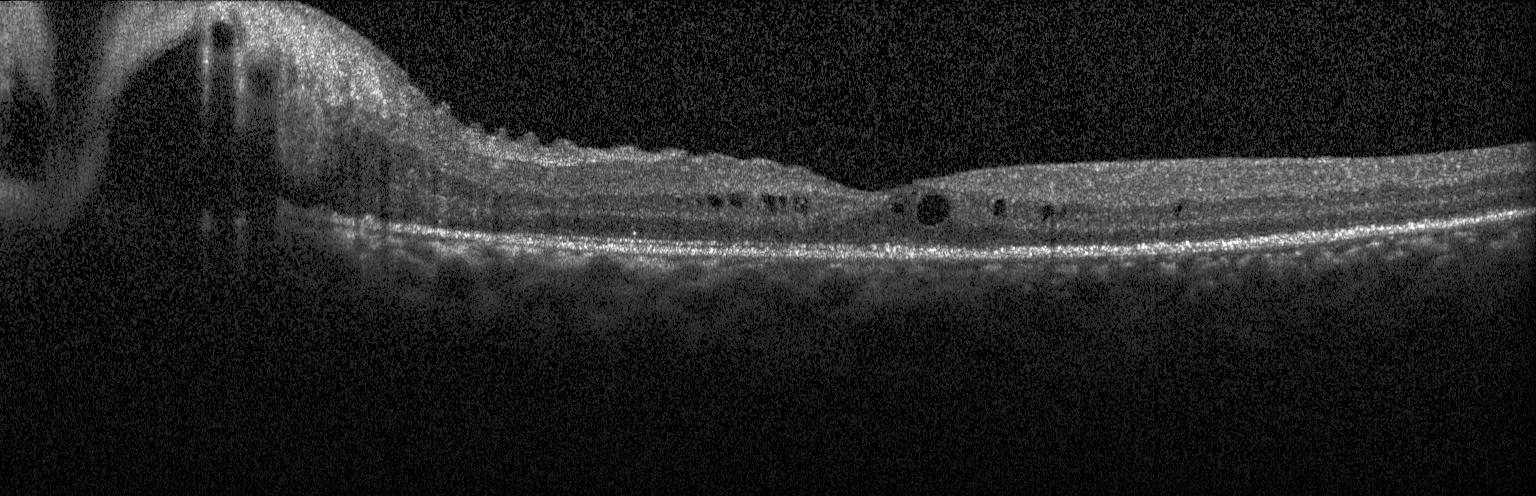
Optical coherence tomography scan.
Diagnosis: DME.